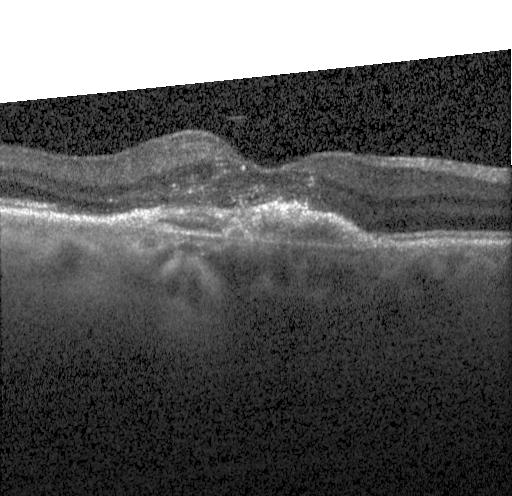
OCT B-scan. Heidelberg Spectralis OCT system
Impression: choroidal neovascularization.